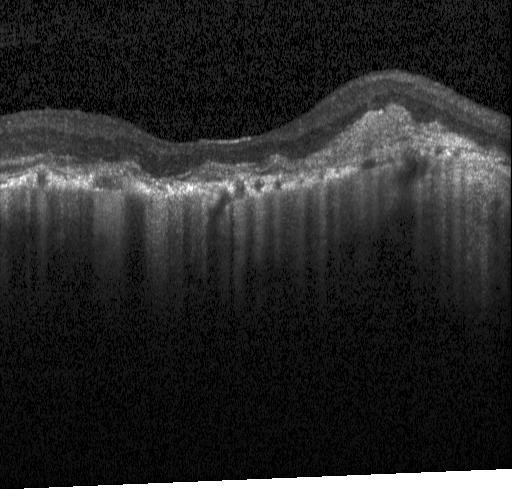

Optical coherence tomography scan, instrument: Heidelberg Spectralis — OCT finding: choroidal neovascularization.